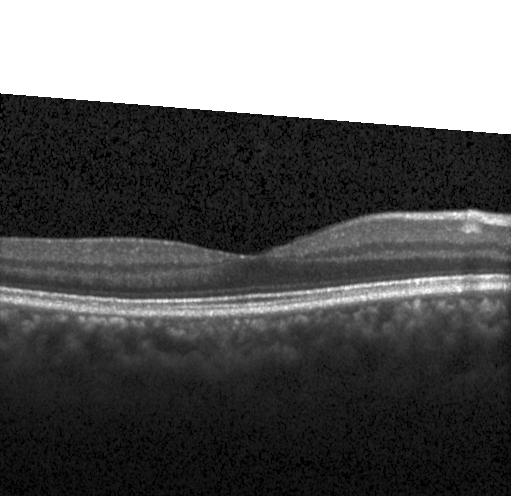 Diagnosis: neither CNV, DME, nor drusen.